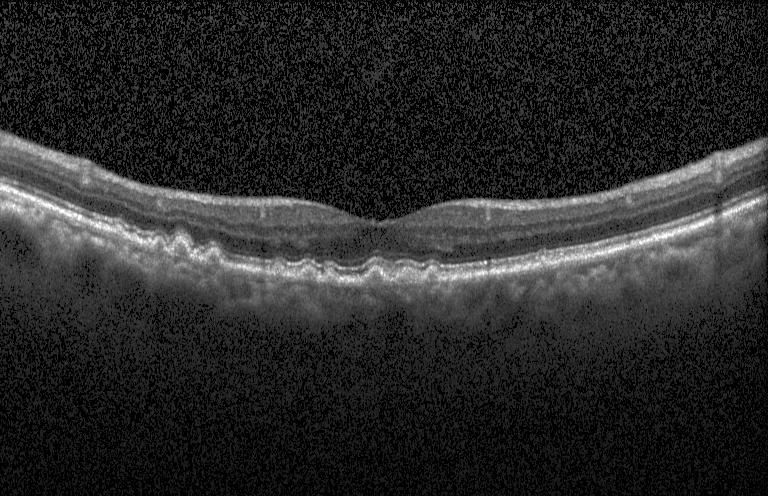

OCT line scan — The scan shows multiple drusen.